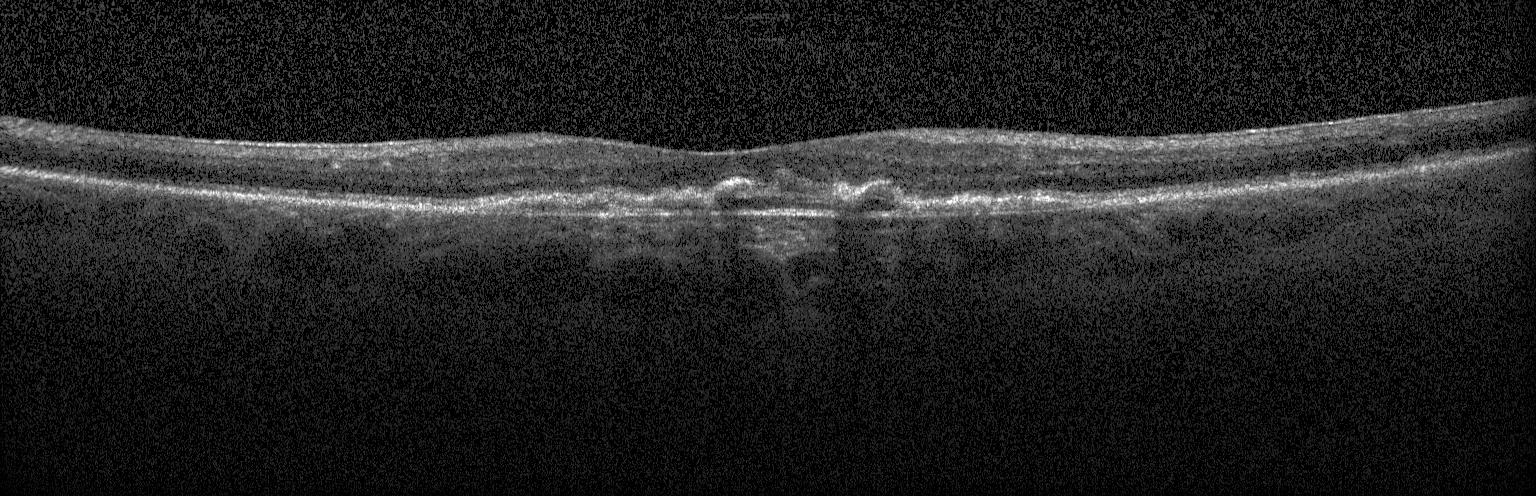

OCT scan showing a choroidal neovascular membrane.